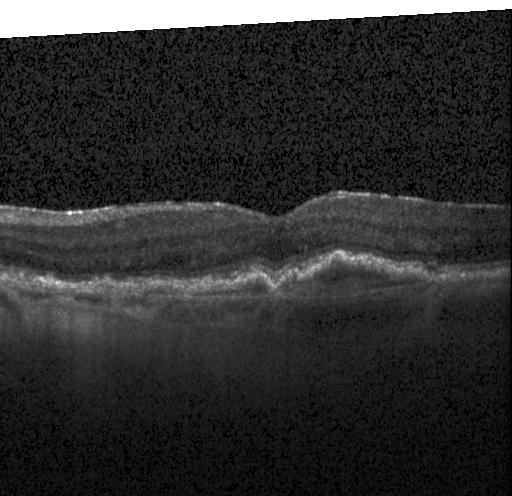 OCT line scan
Choroidal neovascularization.